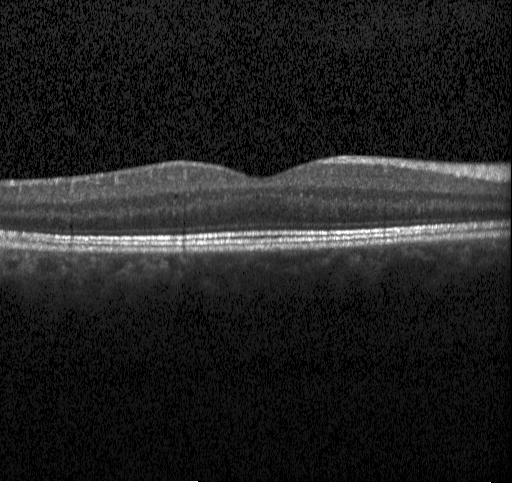
Macular OCT: no choroidal neovascularization, no diabetic macular edema, and no drusen.